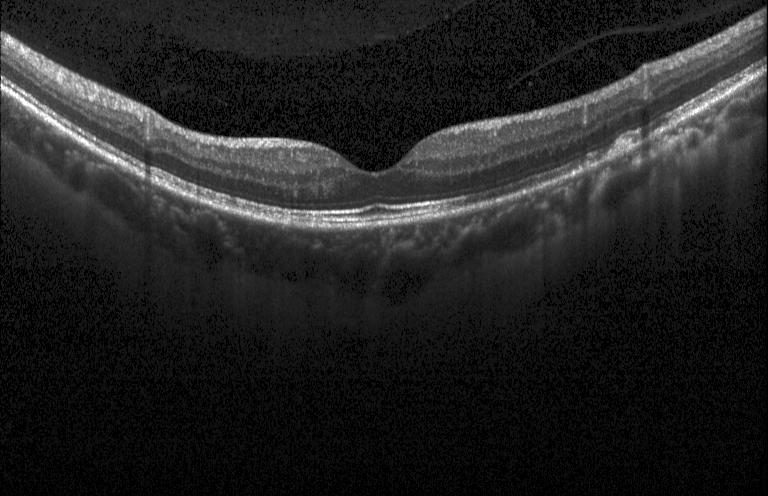 Retinal OCT cross-section — OCT finding: multiple drusen.